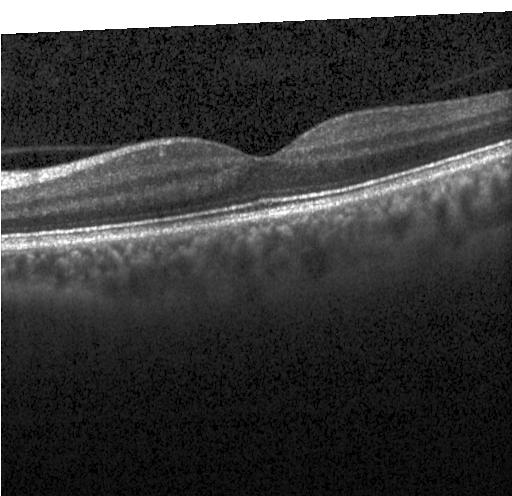

Assessment: no evidence of choroidal neovascularization, diabetic macular edema, or drusen.